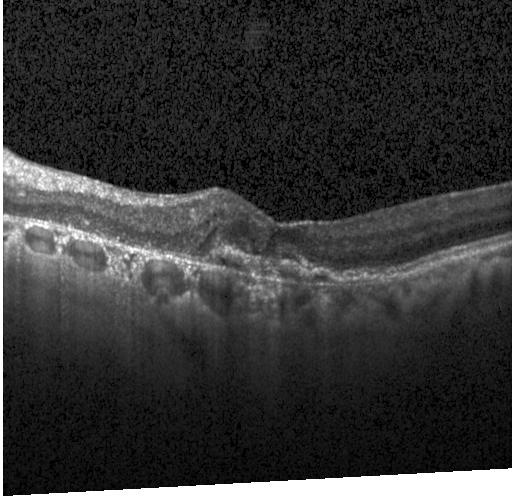

Impression: choroidal neovascularization (CNV).